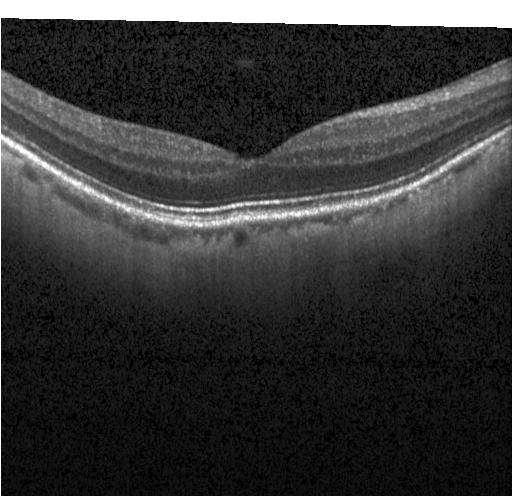 Horizontal scan through the fovea, spectral-domain optical coherence tomography, optical coherence tomography B-scan
Diagnosis: neither CNV, DME, nor drusen.